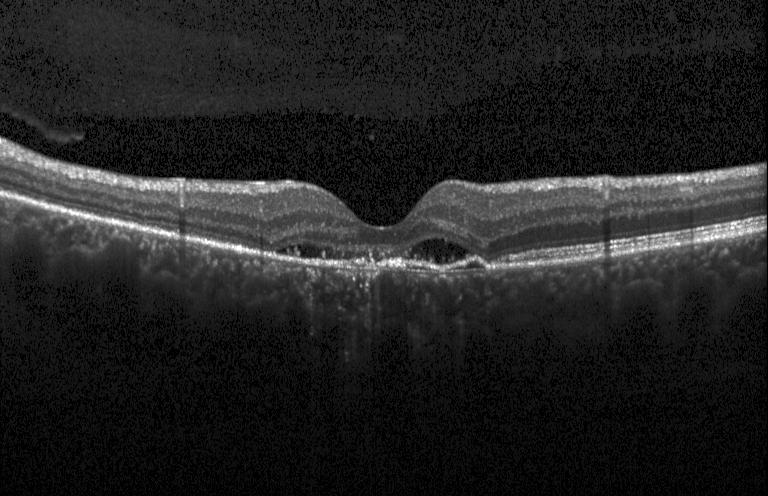
Acquired on a Heidelberg Spectralis; optical coherence tomography scan; spectral-domain OCT — This B-scan demonstrates choroidal neovascularization (CNV).